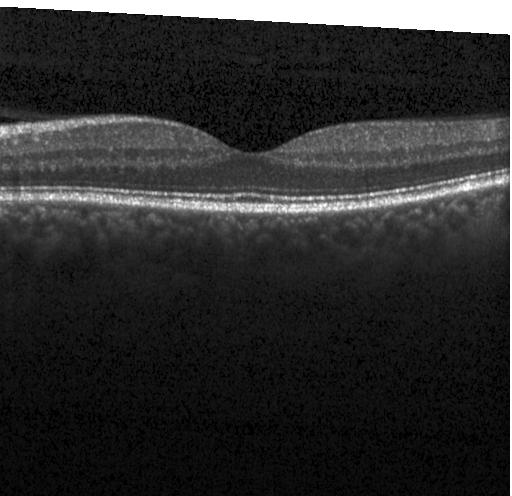 Optical coherence tomography scan · instrument: Heidelberg Spectralis · horizontal scan through the fovea — Dx: no evidence of choroidal neovascularization, diabetic macular edema, or drusen.